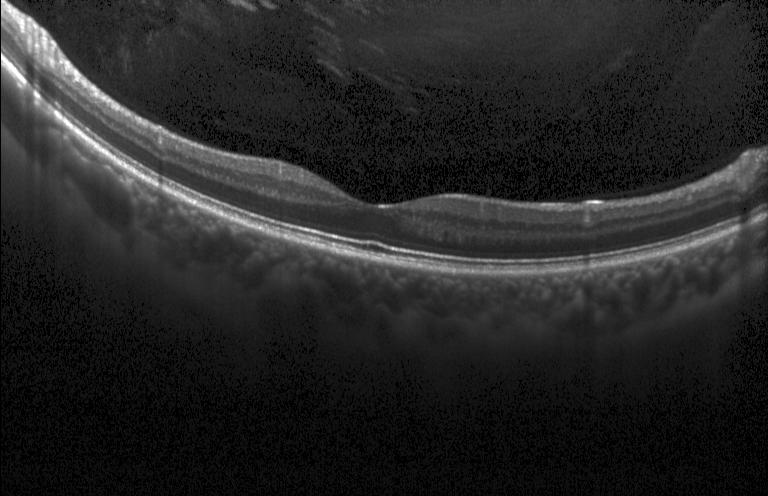

No CNV, no DME, and no drusen.